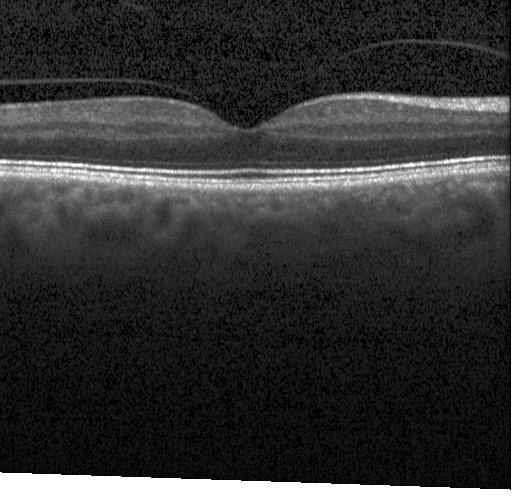

Macular OCT demonstrating no CNV, no DME, and no drusen.